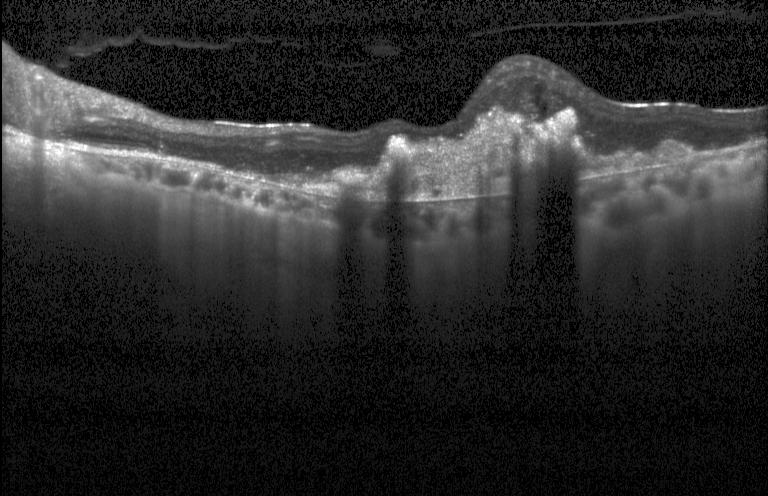

OCT line scan, spectral-domain OCT.
Assessment: a choroidal neovascular membrane.